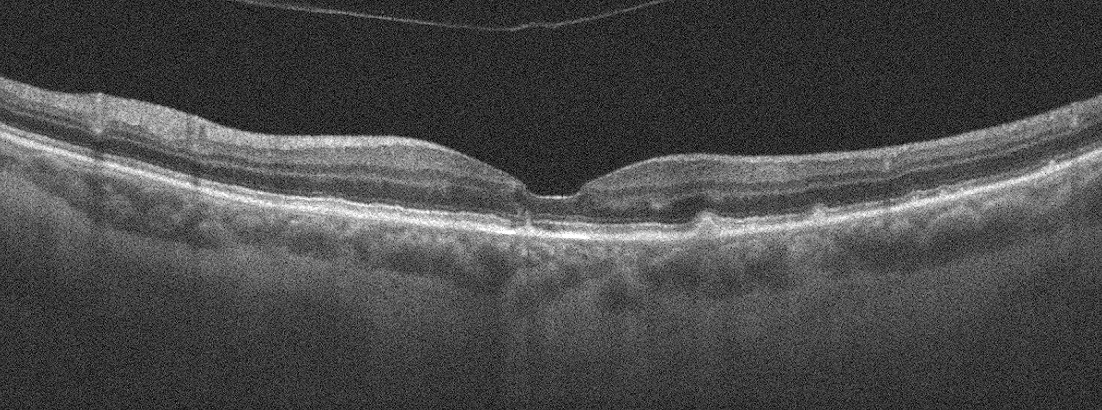 Through the macula. Optovue Avanti RTVue XR. Retinal OCT B-scan. AMD.